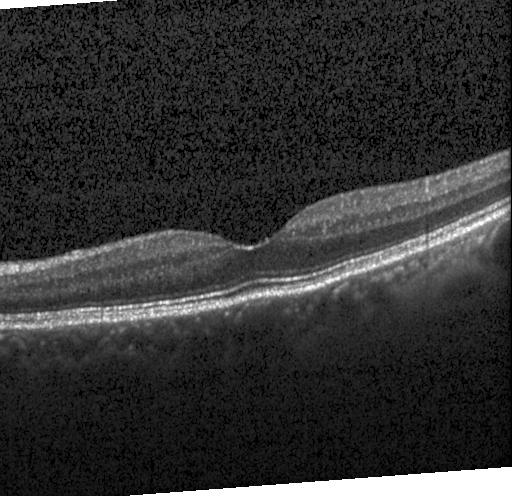

Impression: no choroidal neovascularization, no diabetic macular edema, and no drusen.